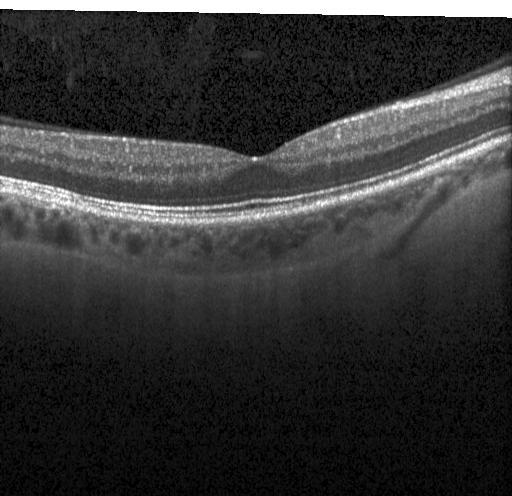
Spectral-domain optical coherence tomography · Heidelberg Spectralis · OCT B-scan · centered on the fovea
This B-scan demonstrates no choroidal neovascularization, diabetic macular edema, or drusen.